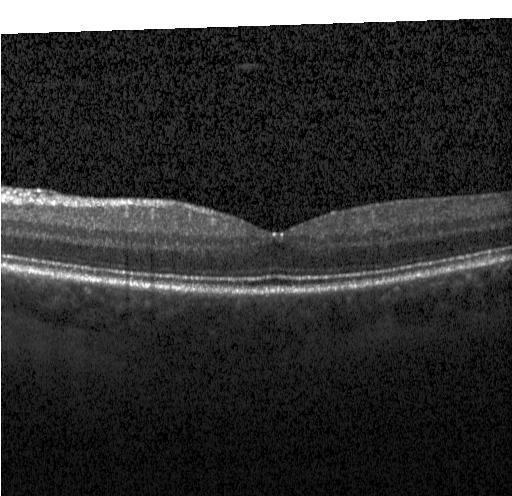 Optical coherence tomography B-scan — Diagnosis: no evidence of choroidal neovascularization, diabetic macular edema, or drusen.